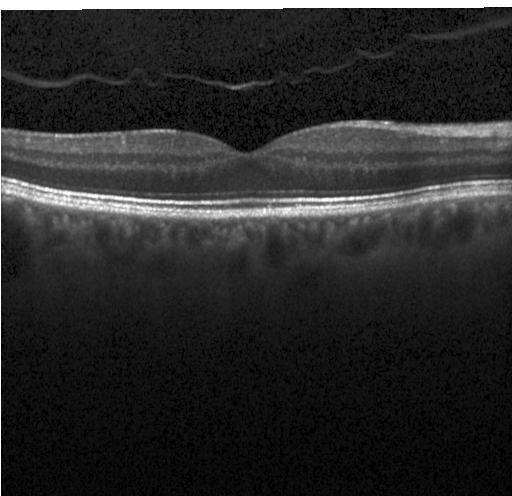

Macular OCT: neither choroidal neovascularization, diabetic macular edema, nor drusen.